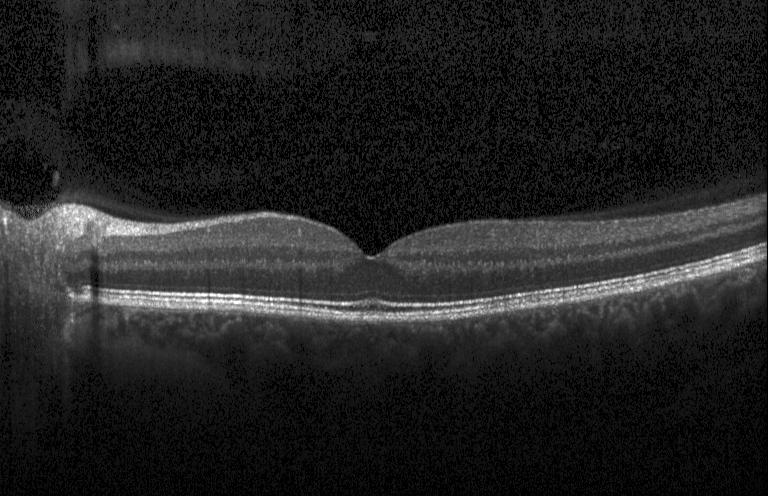

Dx: neither CNV, DME, nor drusen.